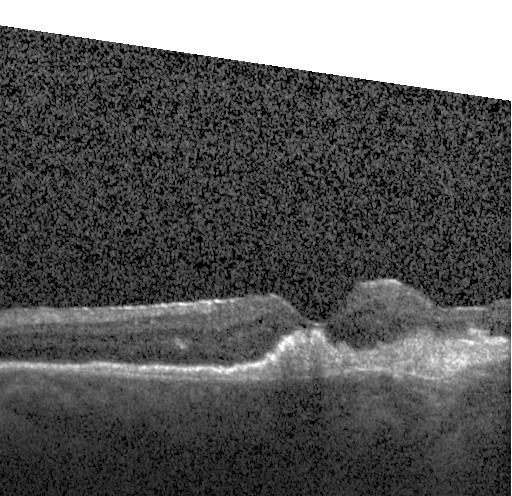

Spectral-domain OCT B-scan: CNV.